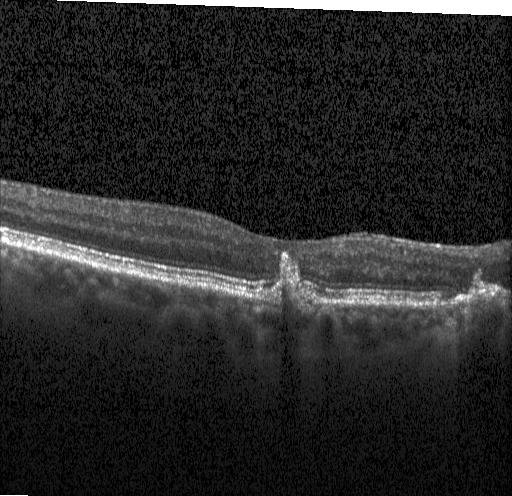

Through the macula. Heidelberg Spectralis OCT system. Spectral-domain OCT. Optical coherence tomography B-scan
Impression: a choroidal neovascular membrane.